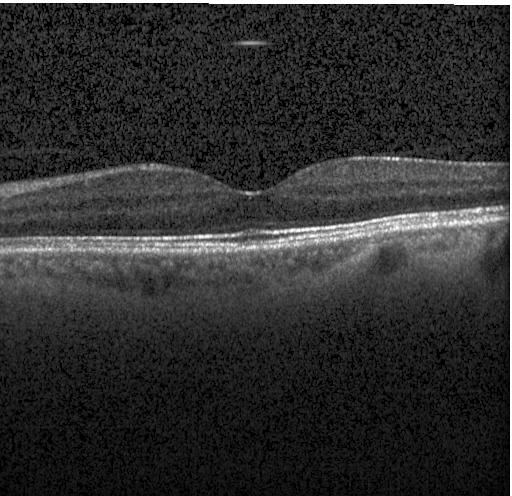
Retinal OCT B-scan. SD-OCT. Finding: no CNV, no DME, and no drusen.